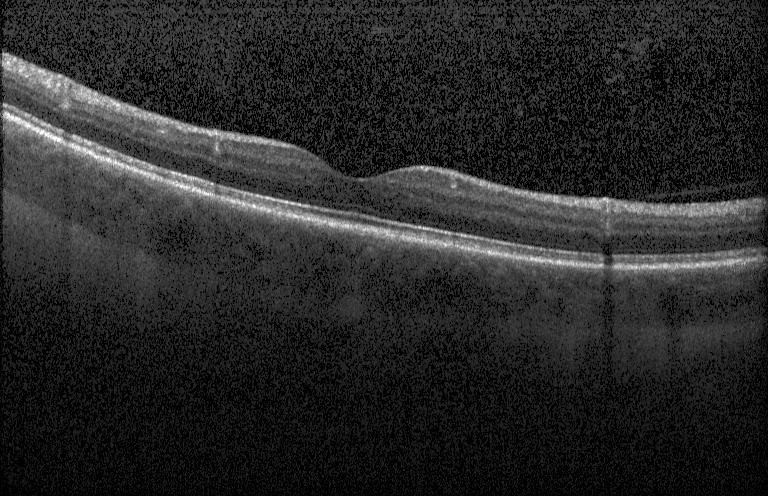 Optical coherence tomography scan; fovea-centered; Heidelberg Spectralis; spectral-domain optical coherence tomography
Finding: neither choroidal neovascularization, diabetic macular edema, nor drusen.